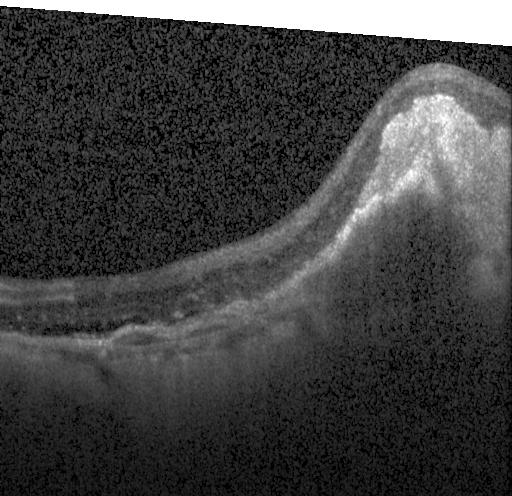

Acquired on a Heidelberg Spectralis · retinal OCT B-scan · spectral-domain optical coherence tomography.
This B-scan demonstrates a choroidal neovascular membrane.